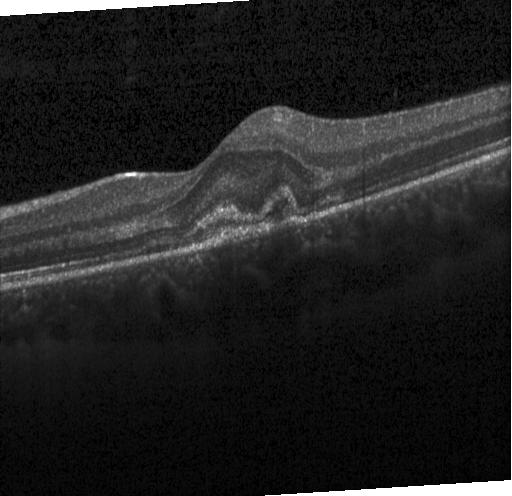
Optical coherence tomography scan · Heidelberg Spectralis
Diagnosis: choroidal neovascularization (CNV).